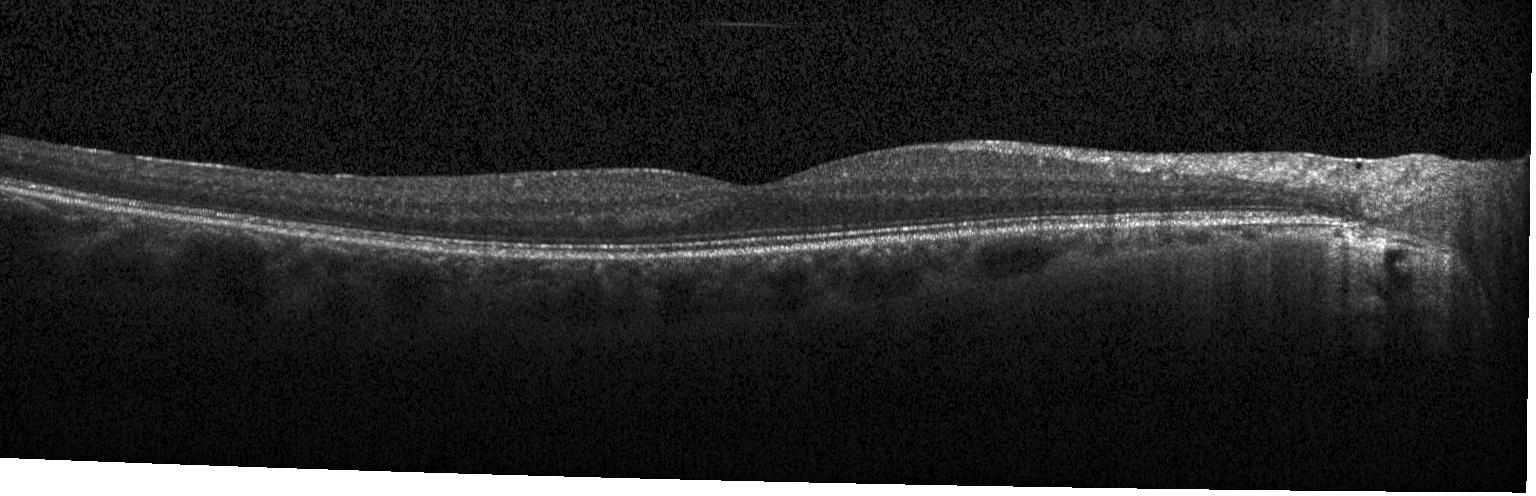 Fovea-centered; OCT line scan; acquired on a Heidelberg Spectralis. Impression: no CNV, DME, or drusen.